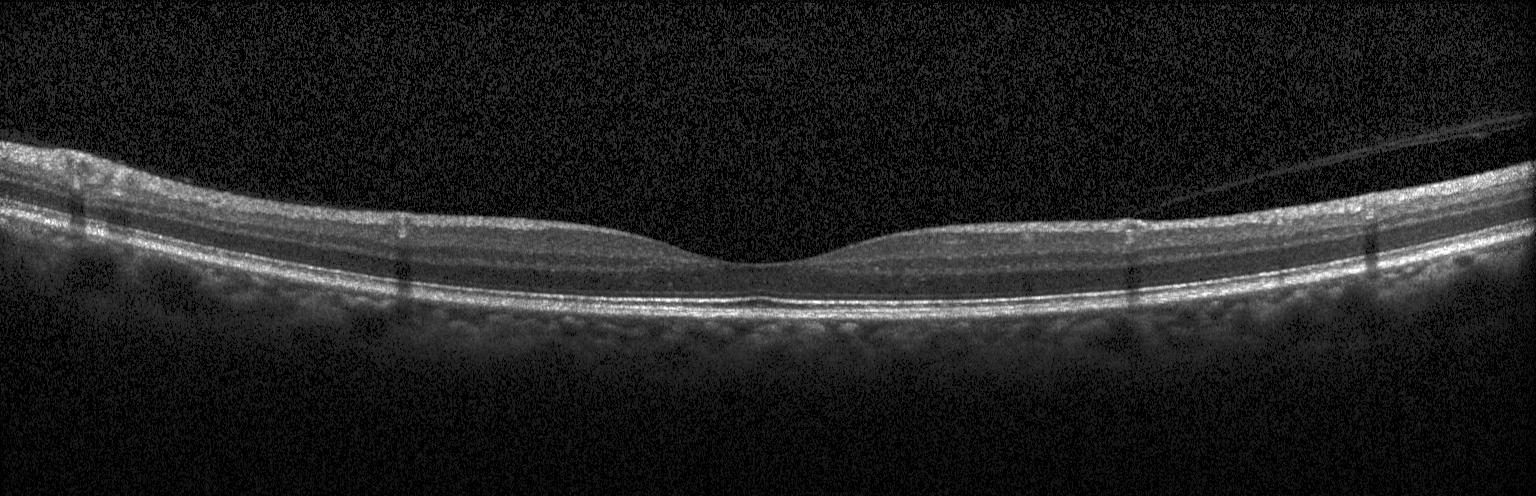
OCT scan showing no evidence of choroidal neovascularization, diabetic macular edema, or drusen.